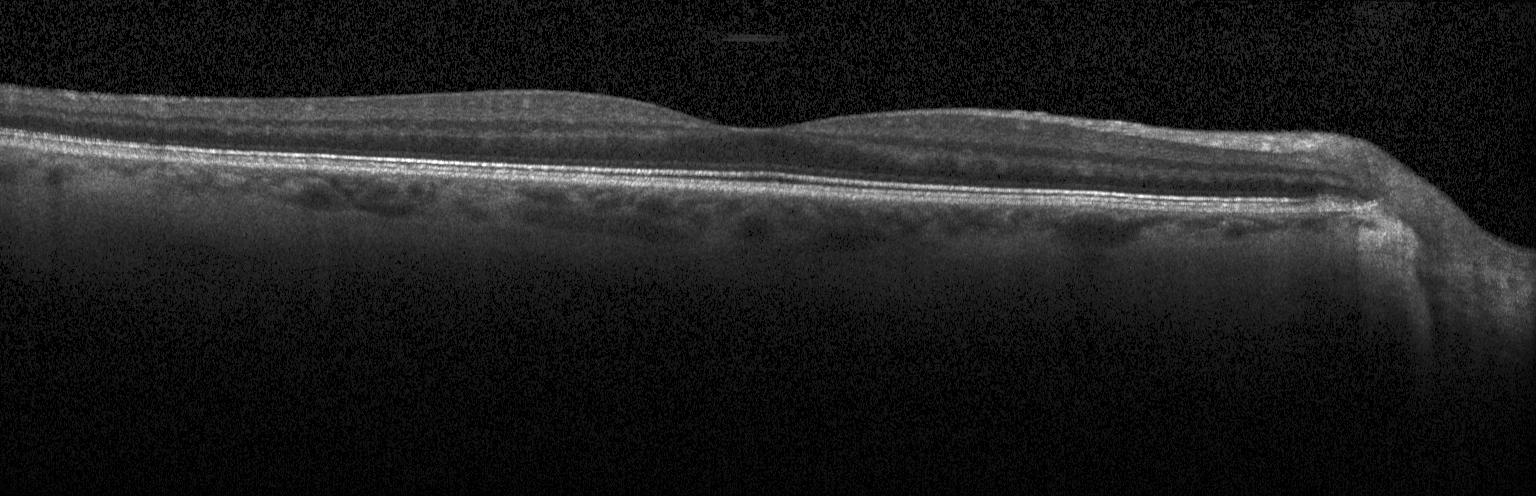 The scan shows no evidence of choroidal neovascularization, diabetic macular edema, or drusen.